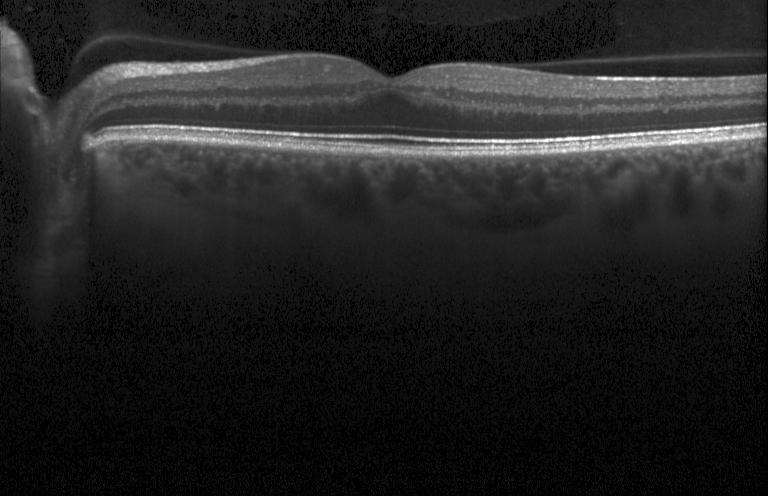 Spectral-domain OCT · macular scan · retinal OCT cross-section · Heidelberg Spectralis OCT system — Assessment: neither CNV, DME, nor drusen.